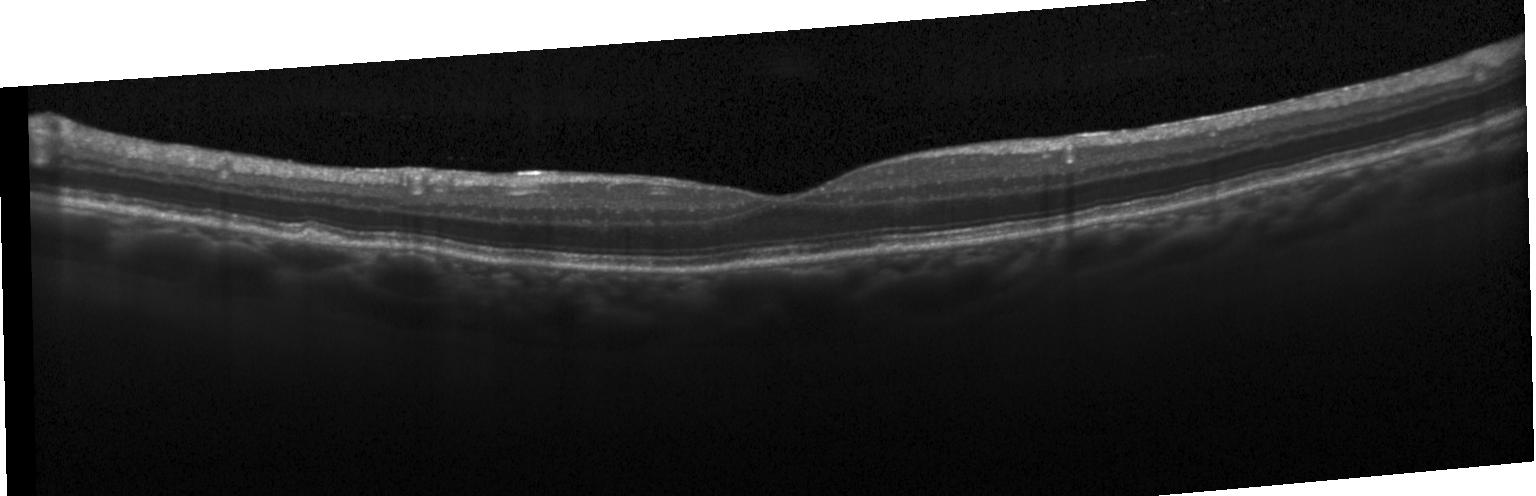

OCT B-scan showing multiple drusen.